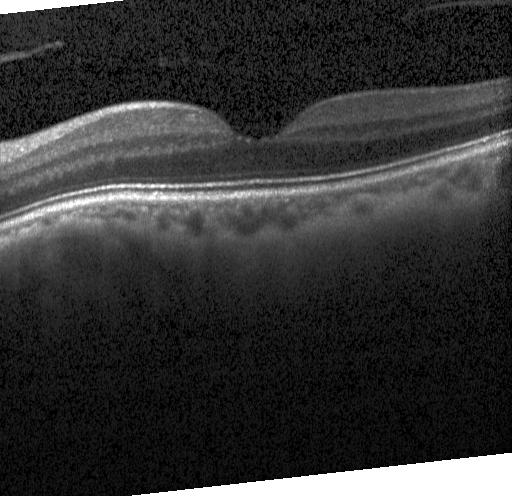 SD-OCT, horizontal scan through the fovea, optical coherence tomography scan.
Diagnosis: no evidence of CNV, DME, or drusen.